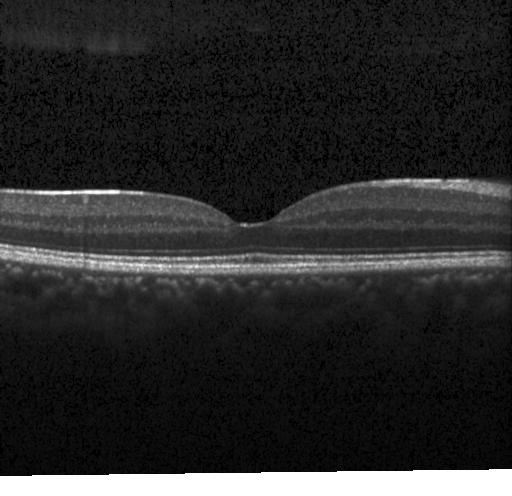 OCT B-scan — The scan shows neither choroidal neovascularization, diabetic macular edema, nor drusen.